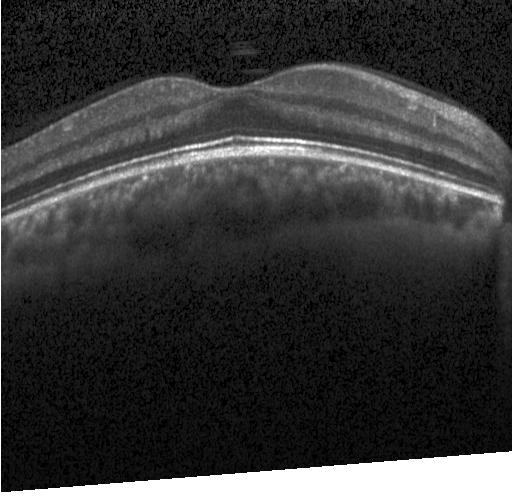
Optical coherence tomography scan. Macular scan — The scan shows no CNV, no DME, and no drusen.